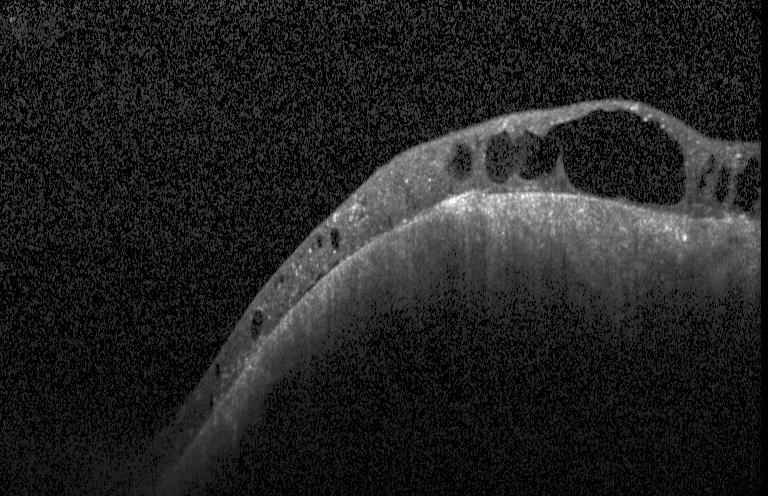 Finding: DME.